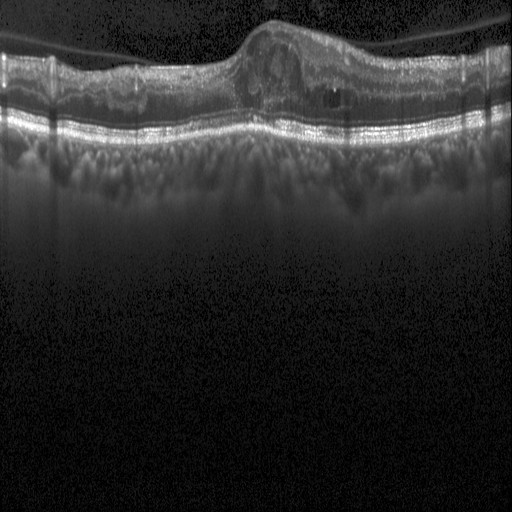
Horizontal scan through the fovea; retinal OCT B-scan; acquired on a Heidelberg Spectralis; spectral-domain optical coherence tomography. Impression: diabetic macular edema.